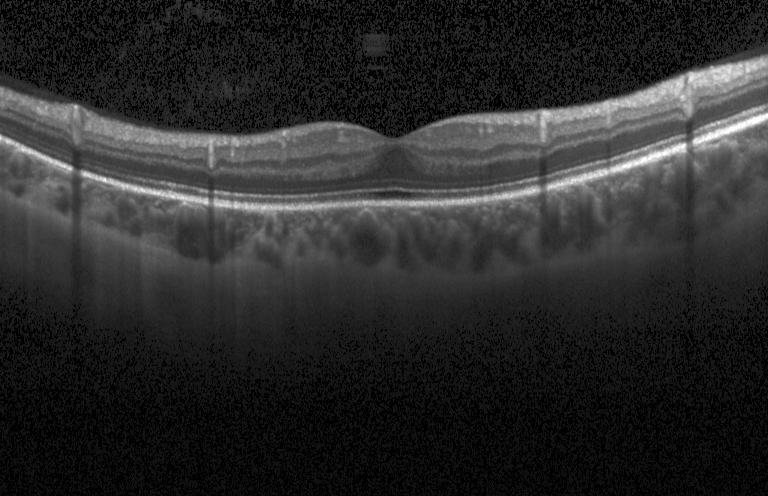

OCT line scan.
No choroidal neovascularization, no diabetic macular edema, and no drusen.